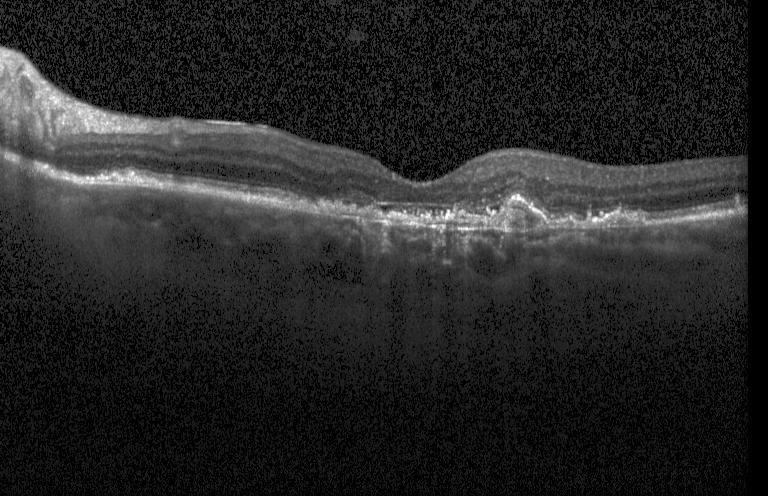 Retinal OCT B-scan. Spectral-domain OCT. Fovea-centered. Instrument: Heidelberg Spectralis. Impression: CNV.